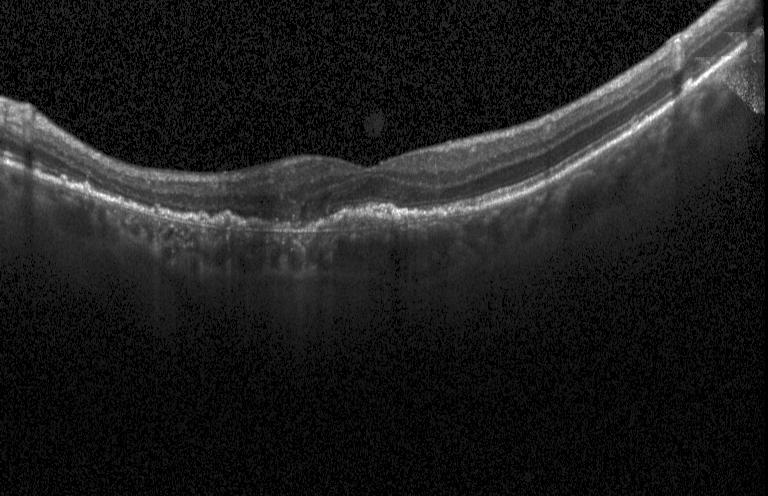

OCT B-scan showing a choroidal neovascular membrane.